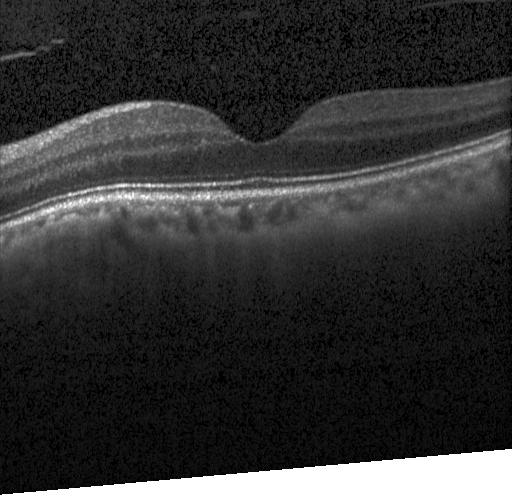 Centered on the fovea; OCT B-scan; spectral-domain OCT; instrument: Heidelberg Spectralis
Impression: no choroidal neovascularization, no diabetic macular edema, and no drusen.